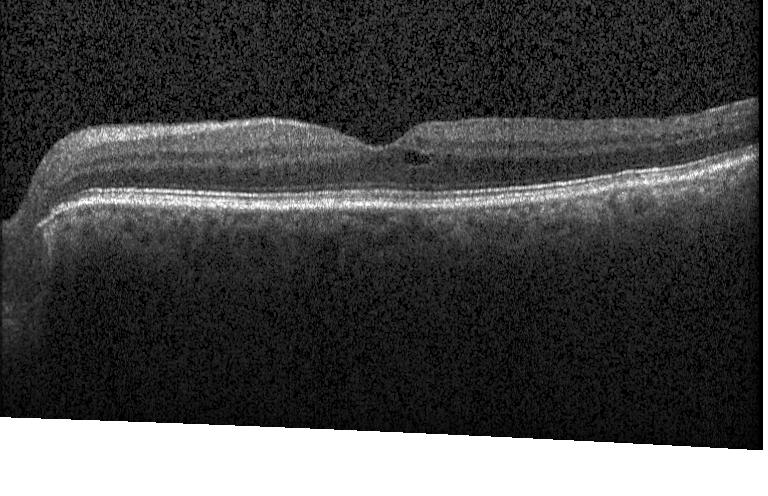
SD-OCT, optical coherence tomography B-scan, Heidelberg Spectralis OCT system.
Impression: DME.